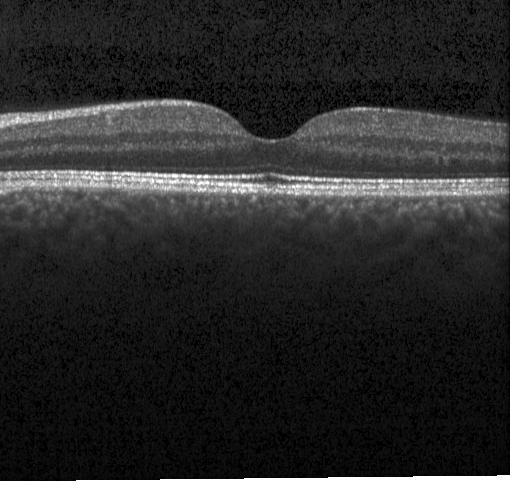 Spectral-domain optical coherence tomography · optical coherence tomography scan · Heidelberg Spectralis OCT system · through the macula.
Diagnosis: no choroidal neovascularization, no diabetic macular edema, and no drusen.